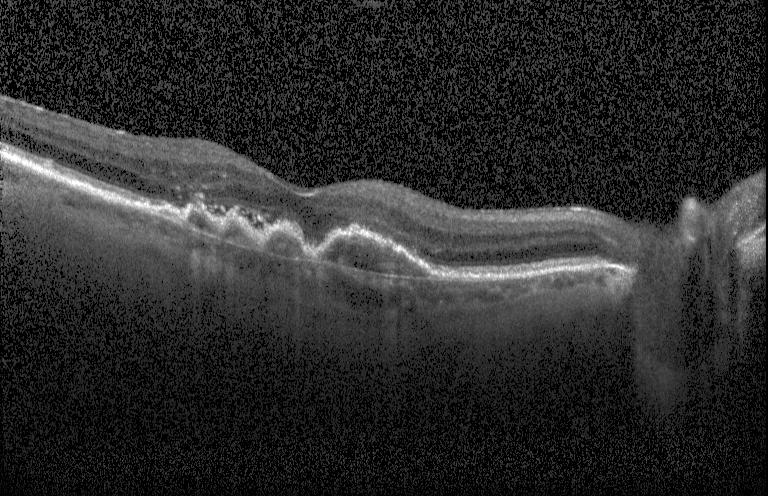 Retinal OCT cross-section; centered on the fovea; Heidelberg Spectralis OCT system
The scan shows a choroidal neovascular membrane.